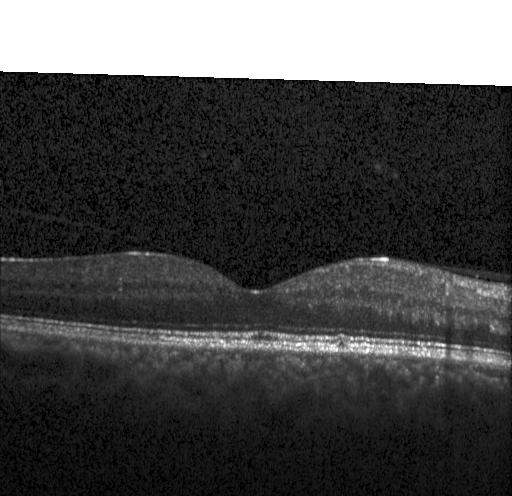 Retinal OCT cross-section, macular scan
This B-scan demonstrates drusen.